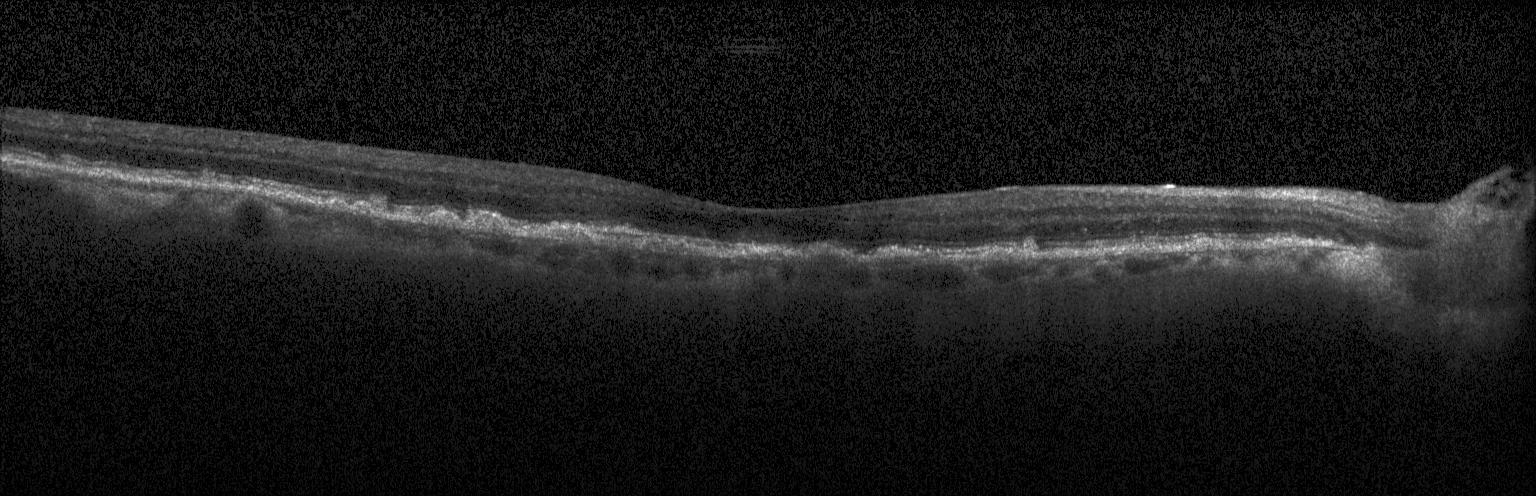 OCT line scan. Diagnosis: a choroidal neovascular membrane.